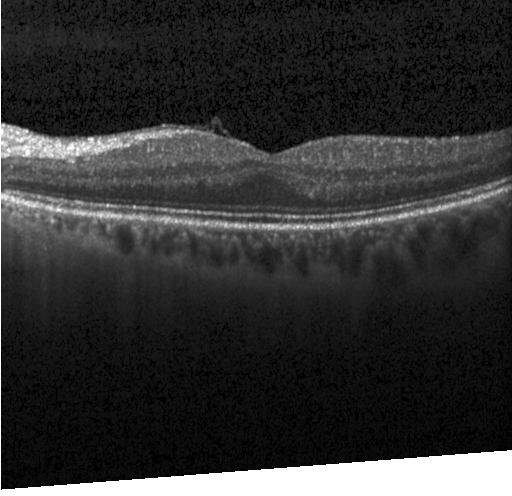

OCT finding: no CNV, no DME, and no drusen.